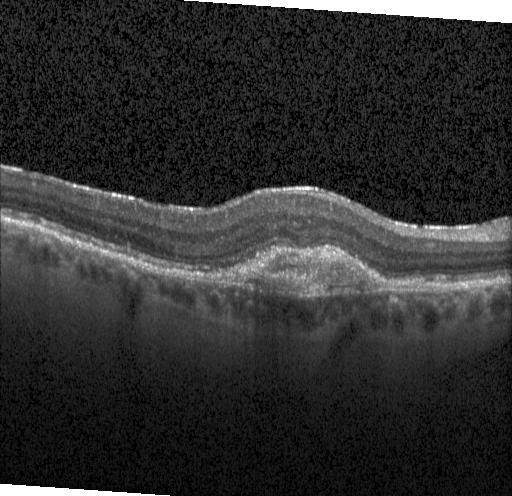 Dx: a choroidal neovascular membrane.